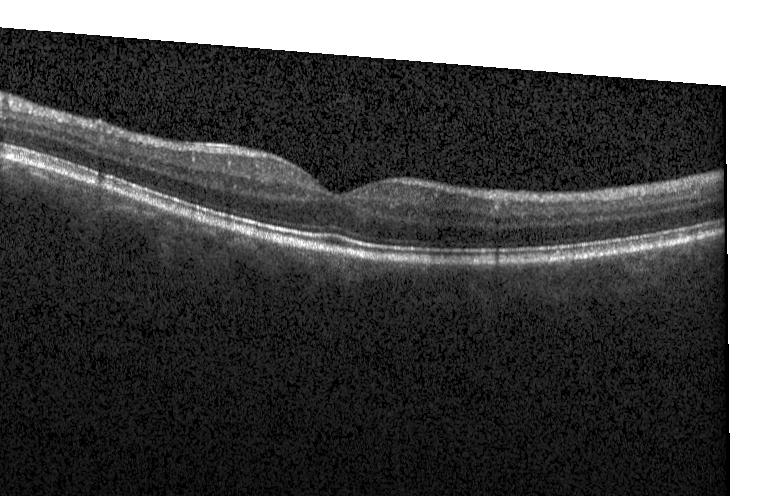 Heidelberg Spectralis · spectral-domain optical coherence tomography · OCT line scan.
Assessment: no evidence of choroidal neovascularization, diabetic macular edema, or drusen.